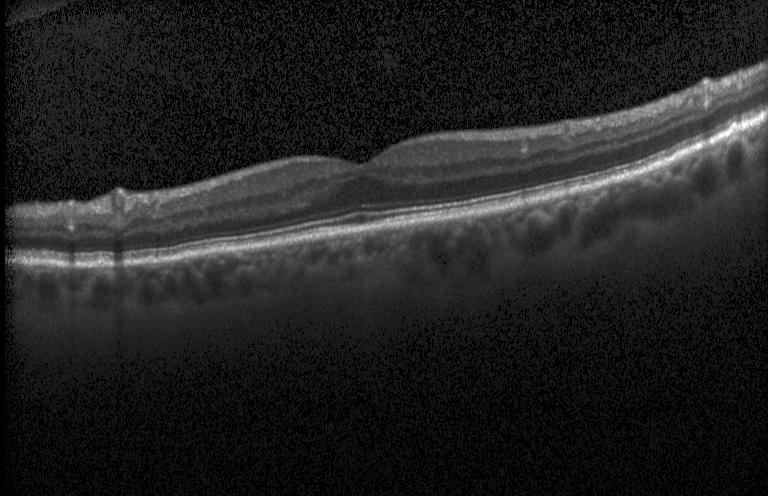

OCT line scan; centered on the fovea. Assessment: no choroidal neovascularization, no diabetic macular edema, and no drusen.